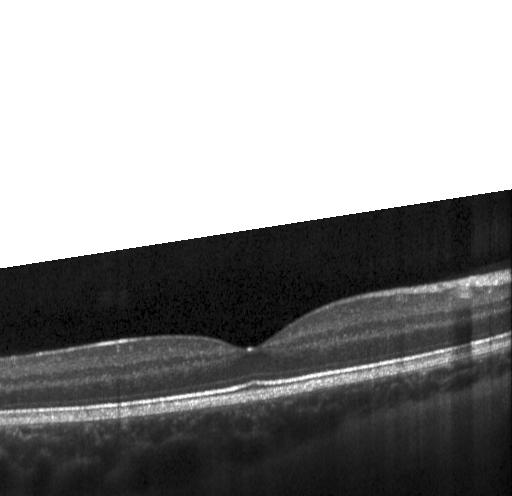
Spectral-domain optical coherence tomography. Retinal OCT cross-section.
Dx: no choroidal neovascularization, no diabetic macular edema, and no drusen.